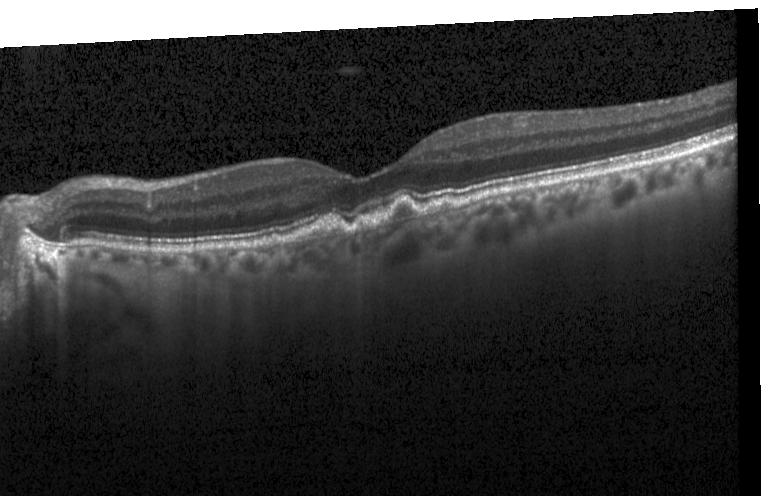 This B-scan demonstrates sub-RPE drusenoid deposits.